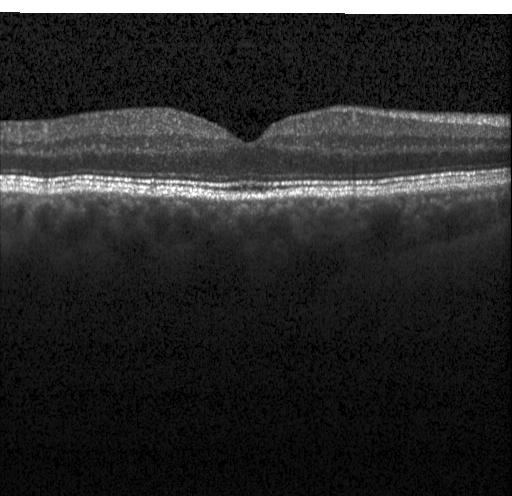

Finding: no evidence of choroidal neovascularization, diabetic macular edema, or drusen.